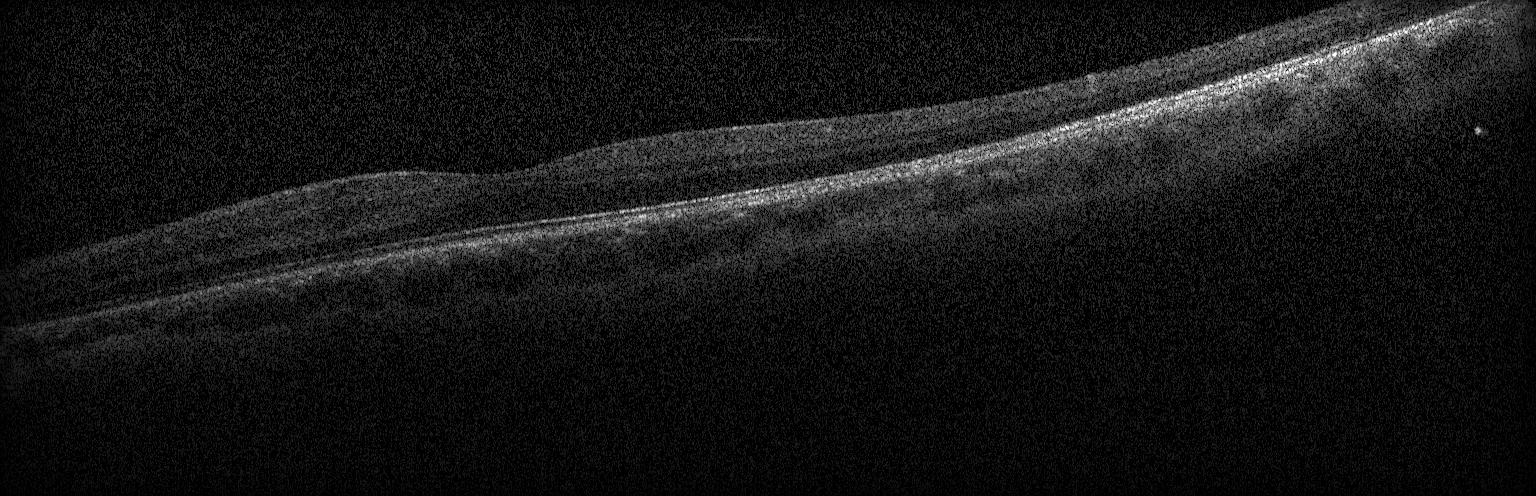

Spectral-domain optical coherence tomography · retinal OCT cross-section · Heidelberg Spectralis · through the macula — Assessment: no CNV, no DME, and no drusen.